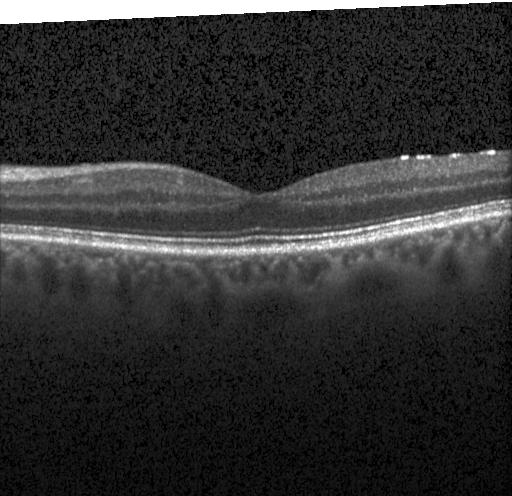 Impression: no evidence of choroidal neovascularization, diabetic macular edema, or drusen.